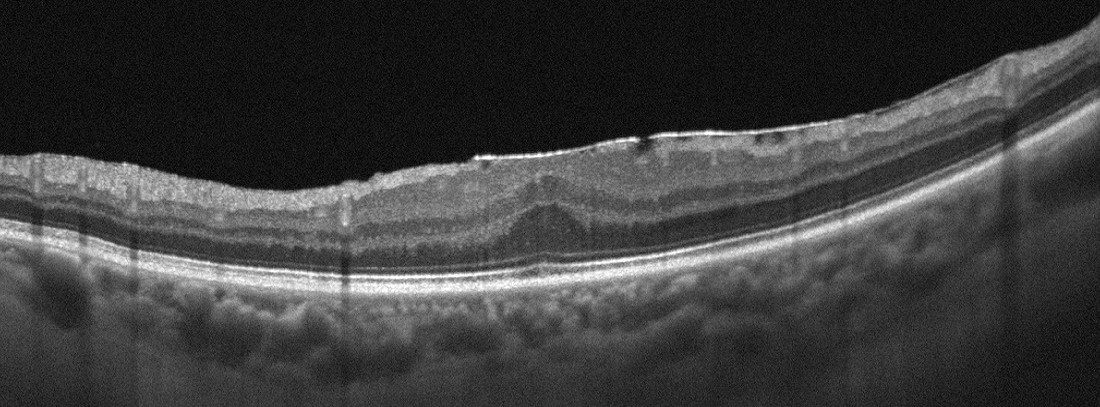 OCT B-scan. Epiretinal membrane.